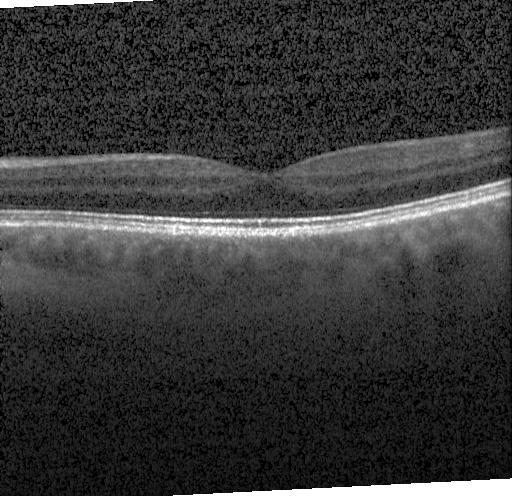

Spectral-domain OCT; acquired on a Heidelberg Spectralis; optical coherence tomography scan. Dx: no choroidal neovascularization, diabetic macular edema, or drusen.